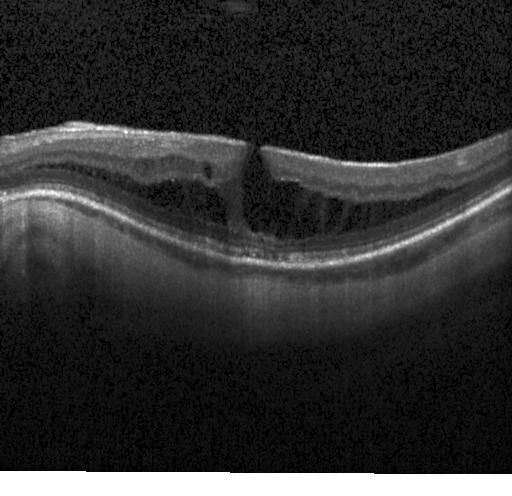
OCT B-scan — OCT finding: diabetic macular edema.